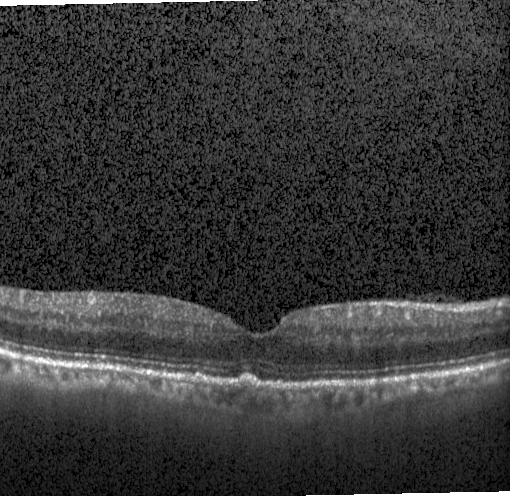 Spectral-domain OCT. Retinal OCT B-scan
Sub-RPE drusenoid deposits.